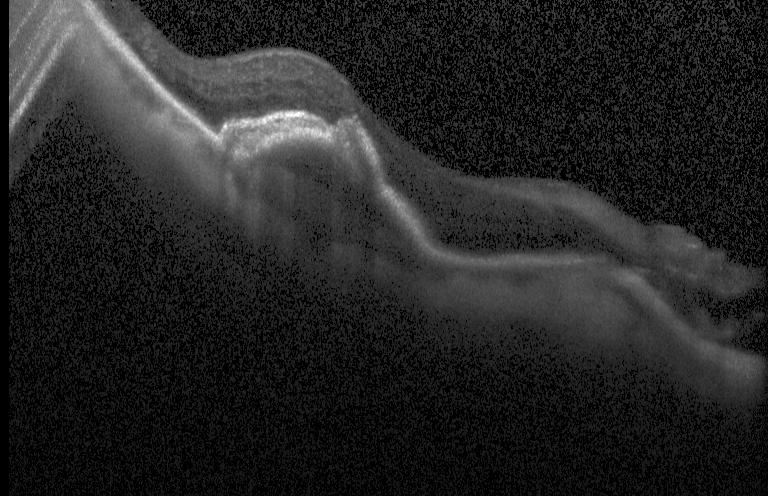
This B-scan demonstrates a choroidal neovascular membrane.